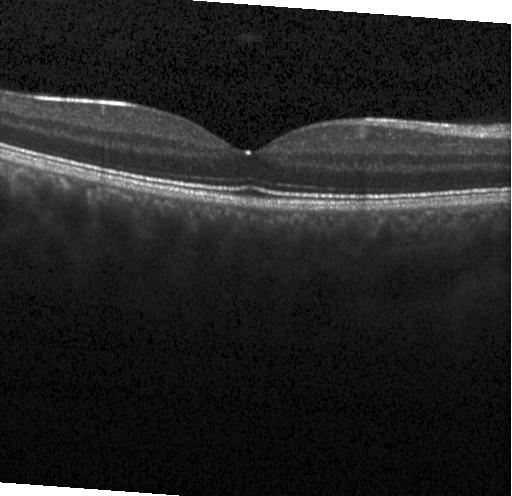
Diagnosis: neither choroidal neovascularization, diabetic macular edema, nor drusen.